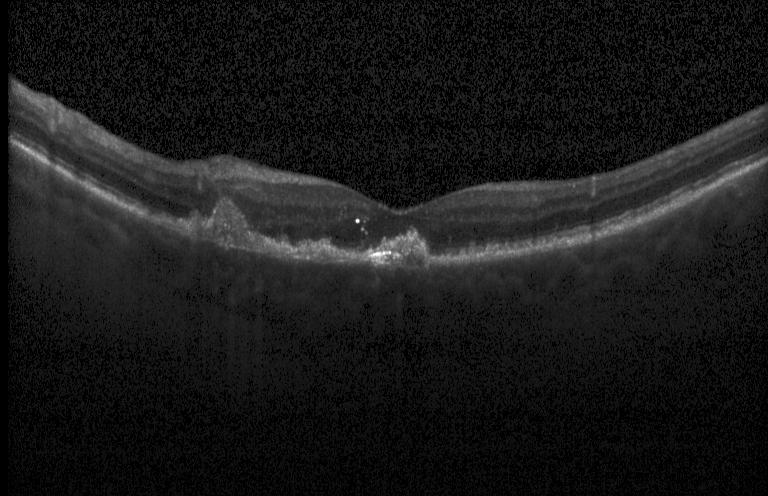 Centered on the fovea; spectral-domain OCT; instrument: Heidelberg Spectralis; retinal OCT cross-section.
Diagnosis: a choroidal neovascular membrane.